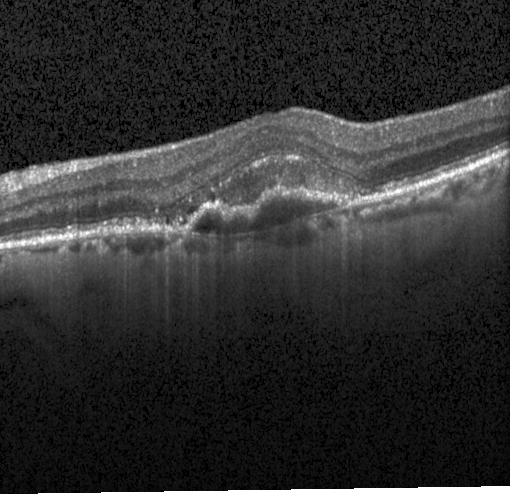
Optical coherence tomography scan · instrument: Heidelberg Spectralis
Impression: a choroidal neovascular membrane.